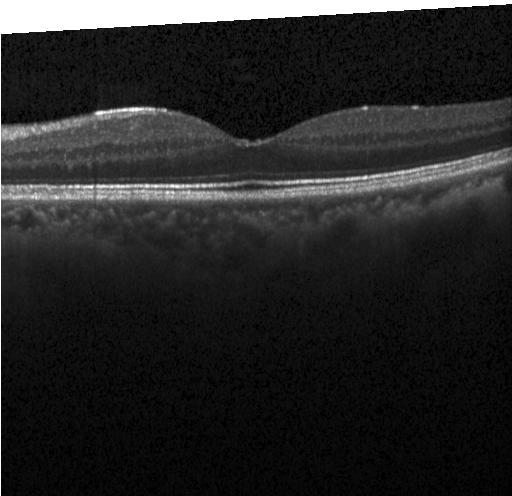
Optical coherence tomography B-scan. No choroidal neovascularization, diabetic macular edema, or drusen.